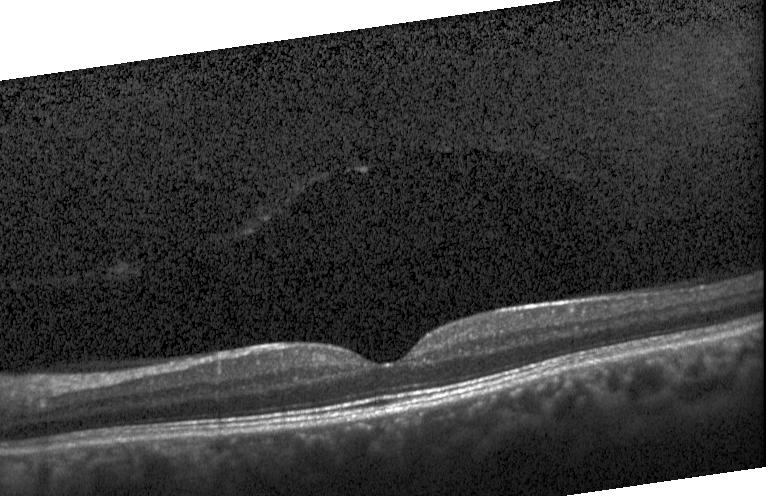 Acquired on a Heidelberg Spectralis · optical coherence tomography scan · fovea-centered · spectral-domain optical coherence tomography. Diagnosis: no evidence of choroidal neovascularization, diabetic macular edema, or drusen.